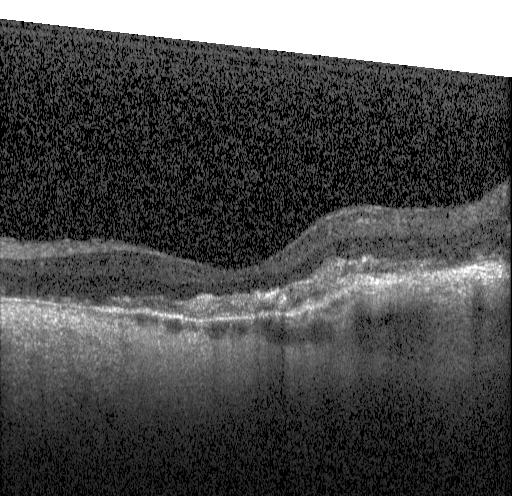

Retinal OCT cross-section. Impression: choroidal neovascularization (CNV).